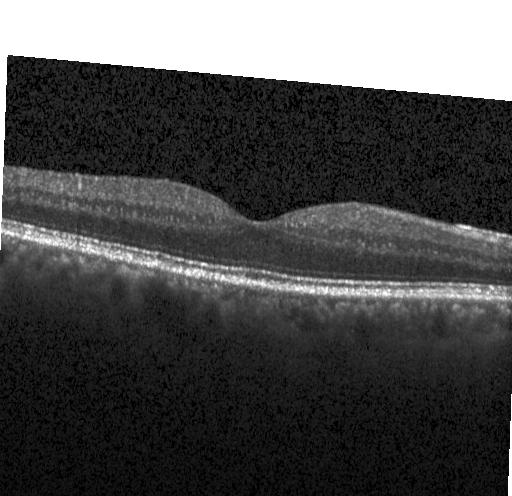 Finding: no evidence of choroidal neovascularization, diabetic macular edema, or drusen.